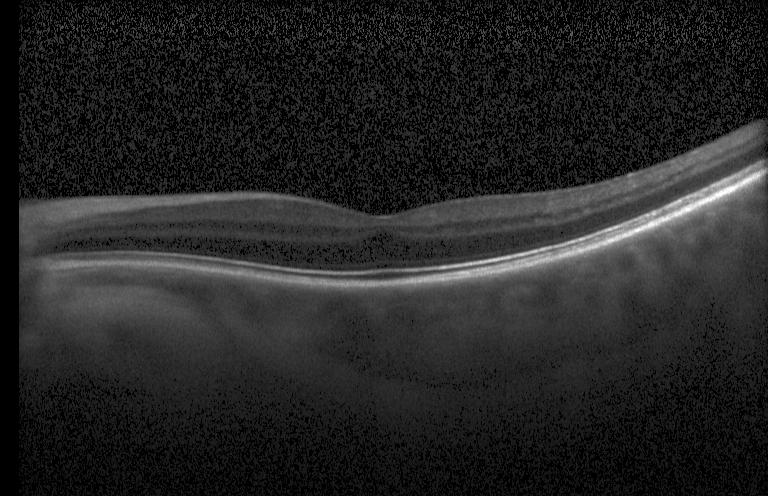 Impression: no CNV, no DME, and no drusen.